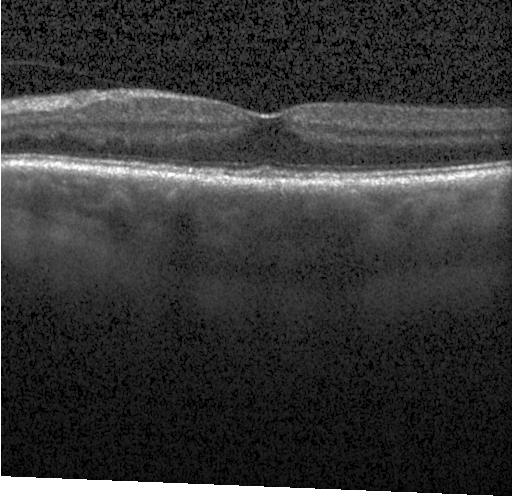
OCT line scan
The scan shows no choroidal neovascularization, no diabetic macular edema, and no drusen.